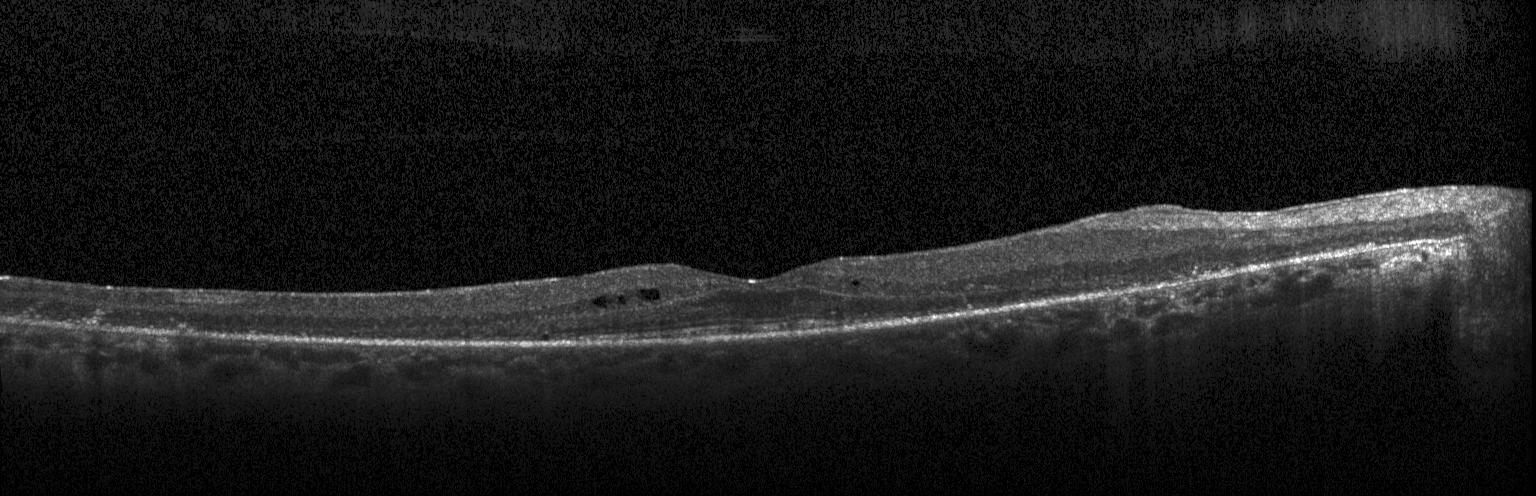

OCT finding: diabetic macular edema (DME).